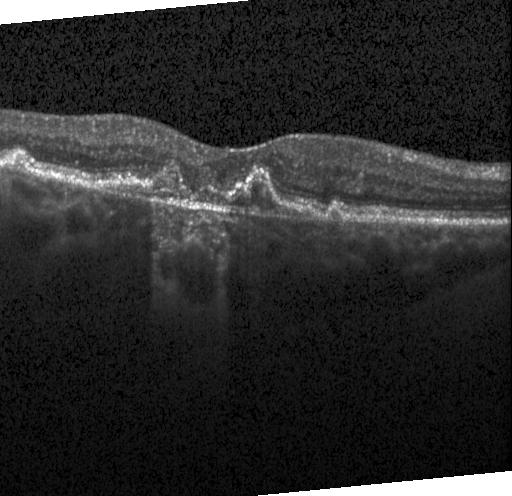

Impression: choroidal neovascularization.